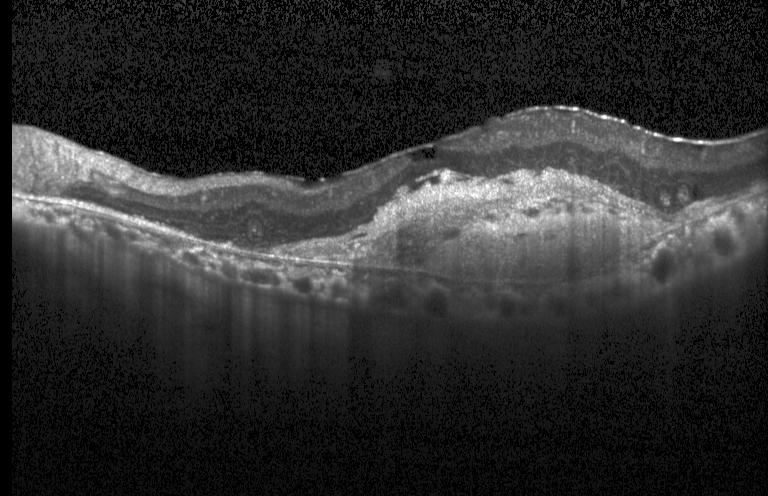
Dx: a choroidal neovascular membrane.